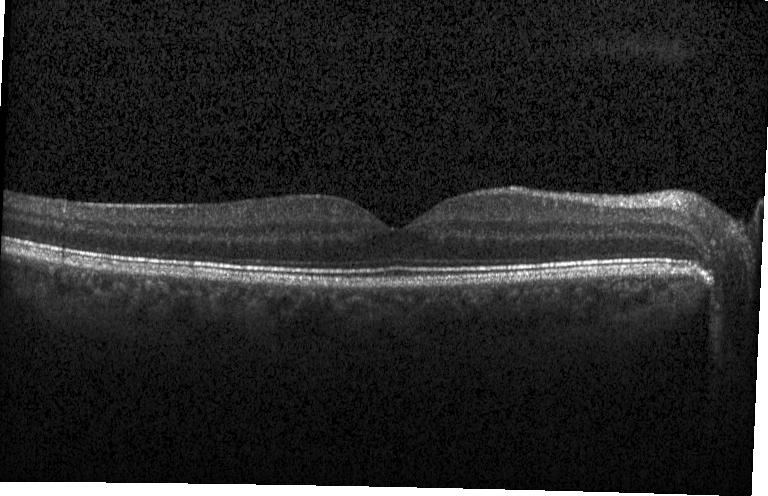

Spectral-domain optical coherence tomography. Fovea-centered. OCT line scan. Acquired on a Heidelberg Spectralis.
Diagnosis: no choroidal neovascularization, diabetic macular edema, or drusen.